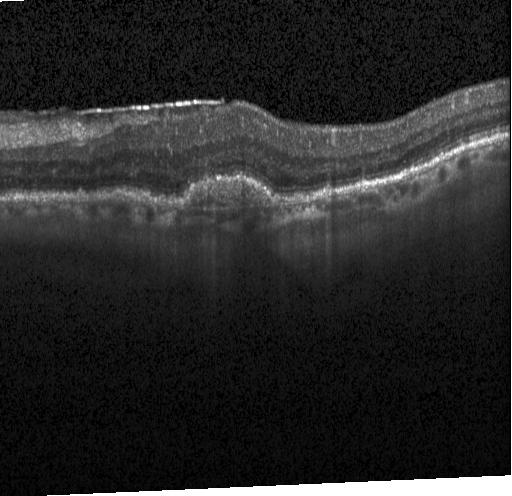 SD-OCT. Optical coherence tomography scan. This B-scan demonstrates choroidal neovascularization.